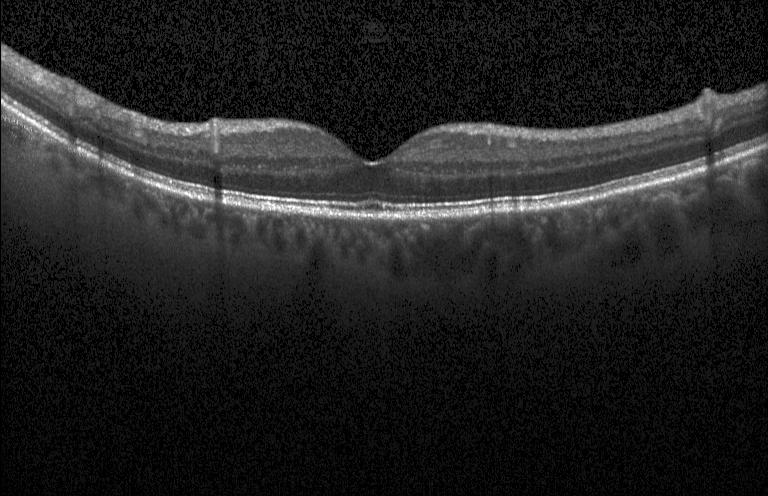
Retinal OCT B-scan. Diagnosis: no evidence of choroidal neovascularization, diabetic macular edema, or drusen.